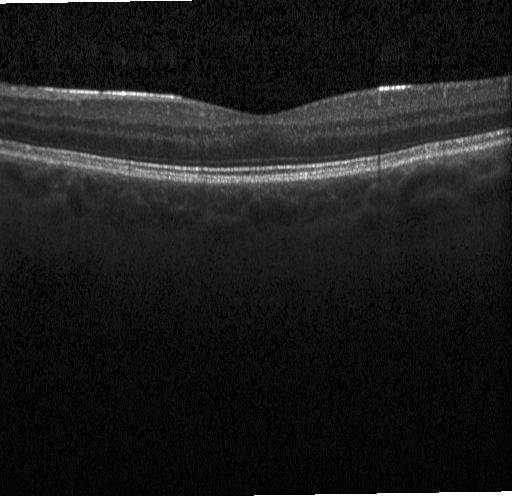 This B-scan demonstrates neither choroidal neovascularization, diabetic macular edema, nor drusen.